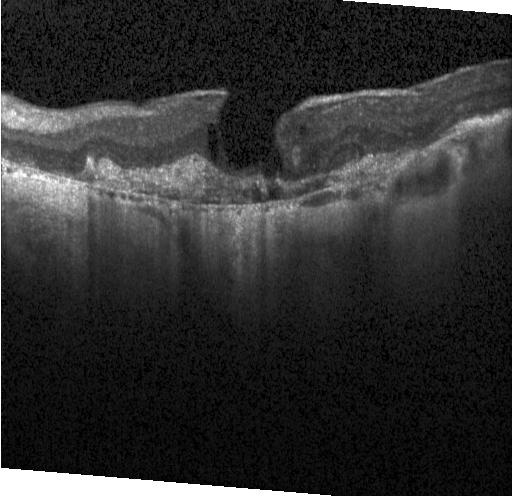
The scan shows choroidal neovascularization.